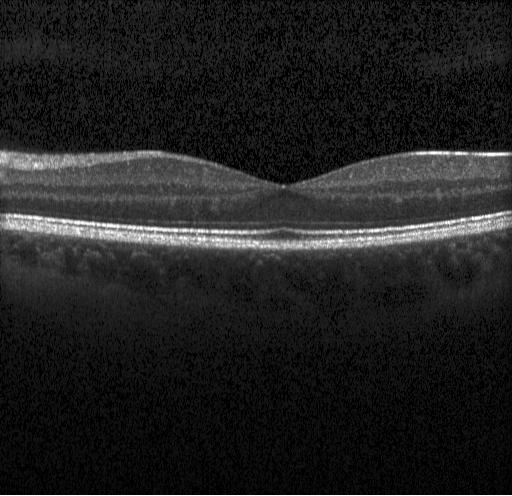 Finding: no CNV, DME, or drusen.